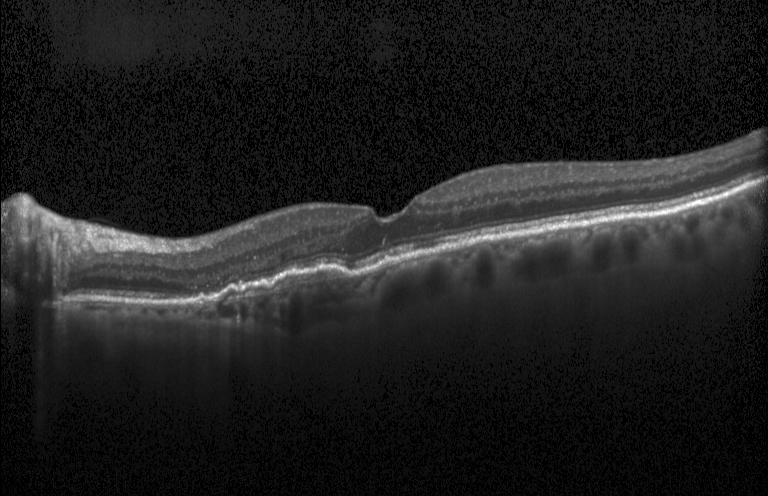

Macular OCT demonstrating a choroidal neovascular membrane.